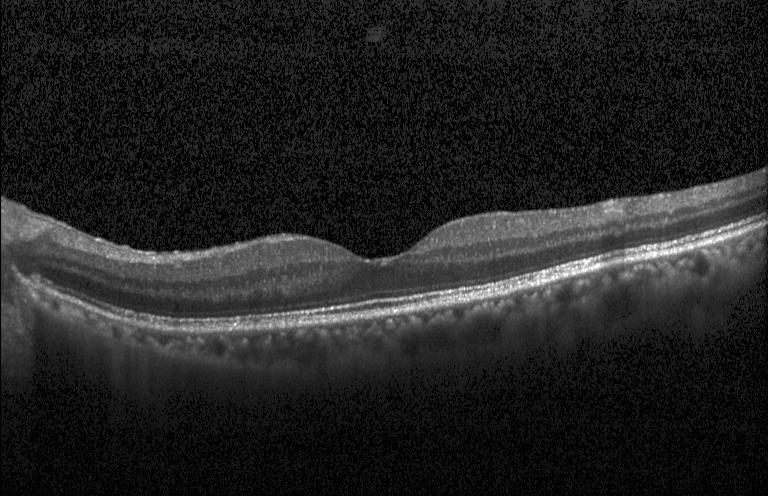
SD-OCT · fovea-centered · acquired on a Heidelberg Spectralis · retinal OCT cross-section.
Finding: neither choroidal neovascularization, diabetic macular edema, nor drusen.